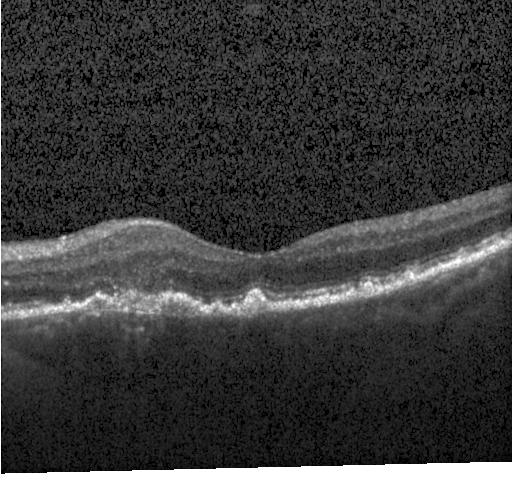 Retinal OCT cross-section showing a choroidal neovascular membrane.